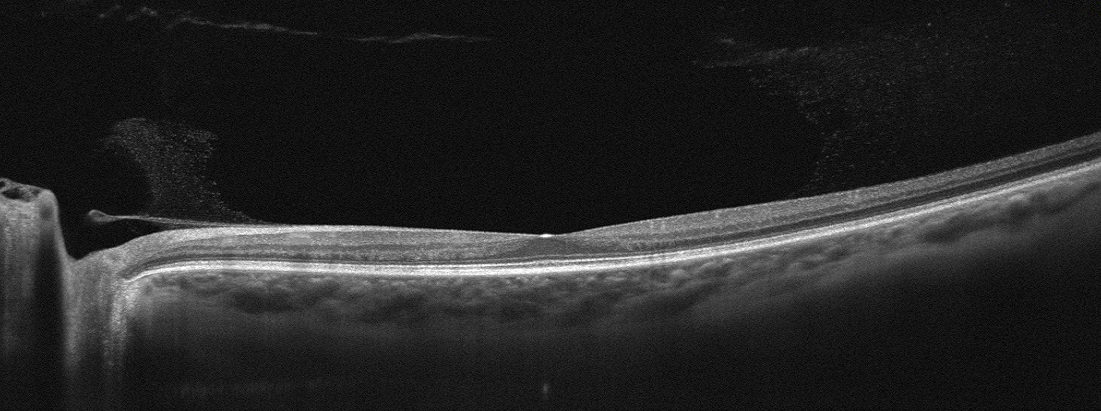

Optovue Avanti RTVue XR; macular scan; retinal OCT B-scan — This B-scan demonstrates no AMD, DME, ERM, RAO, RVO, or VID.